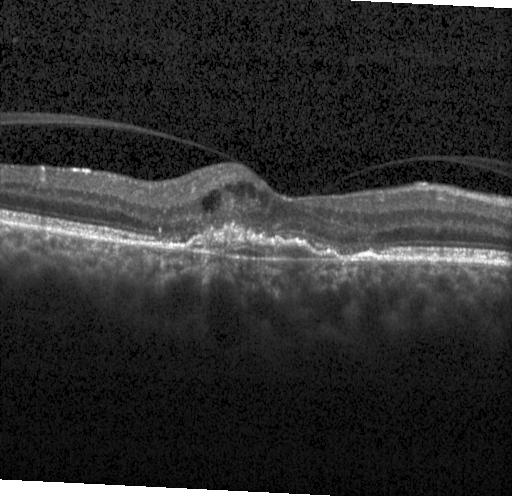

Optical coherence tomography B-scan — OCT finding: choroidal neovascularization.